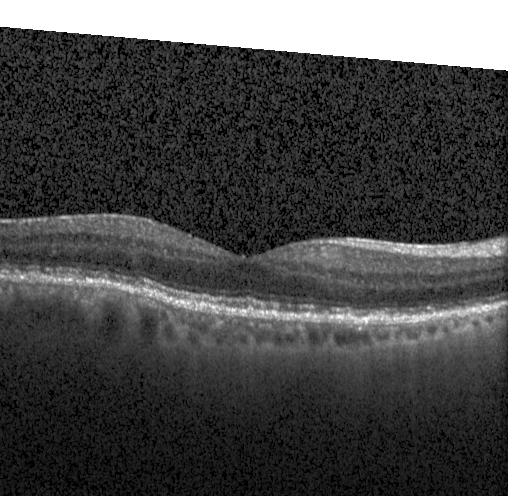
Finding: no evidence of CNV, DME, or drusen.